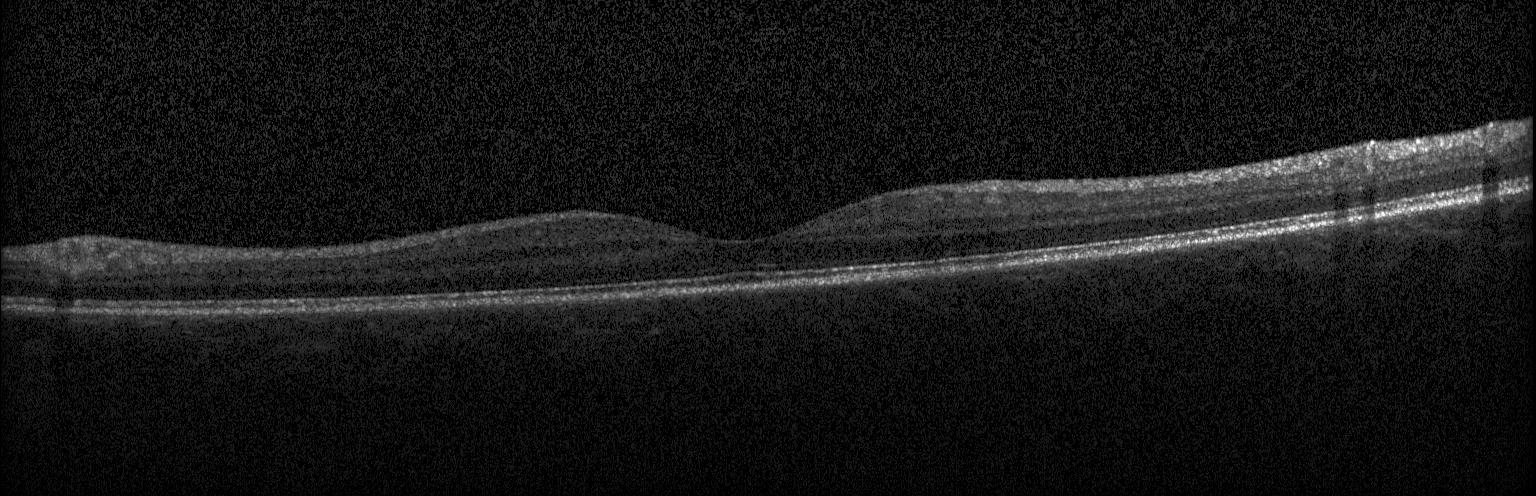
Impression: neither choroidal neovascularization, diabetic macular edema, nor drusen.